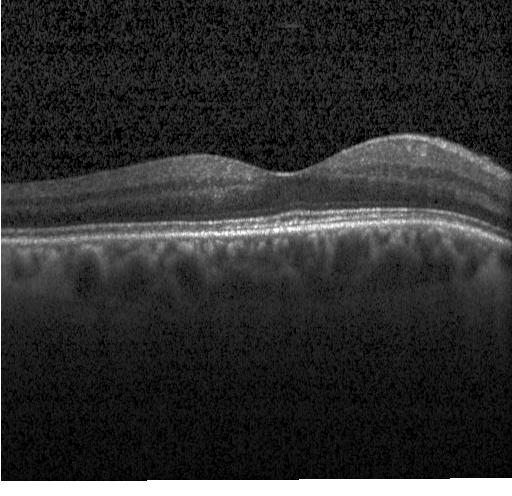

The scan shows neither choroidal neovascularization, diabetic macular edema, nor drusen.